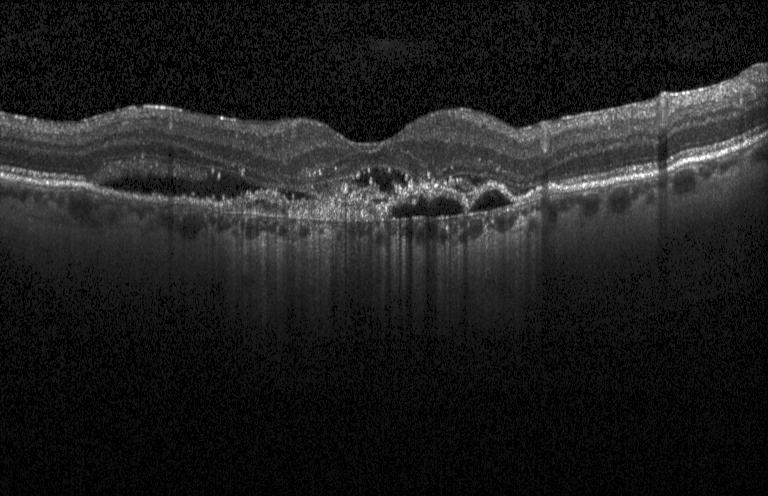
Optical coherence tomography B-scan. Finding: a choroidal neovascular membrane.